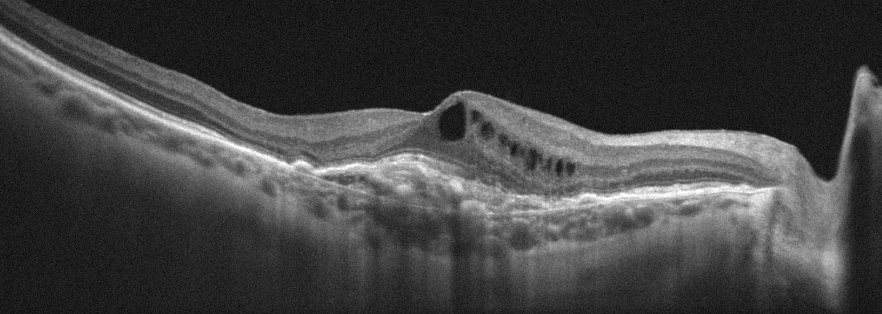
Optical coherence tomography scan, OD. Diagnosis: age-related macular degeneration (AMD).